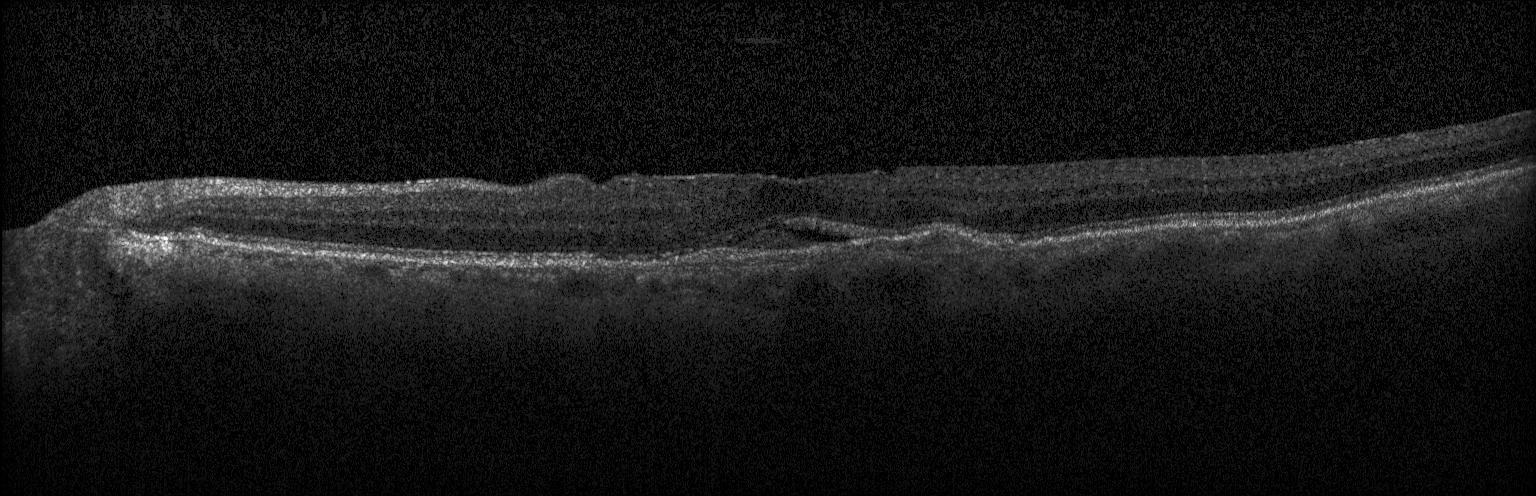 OCT line scan; spectral-domain optical coherence tomography; macular scan. The scan shows a choroidal neovascular membrane.